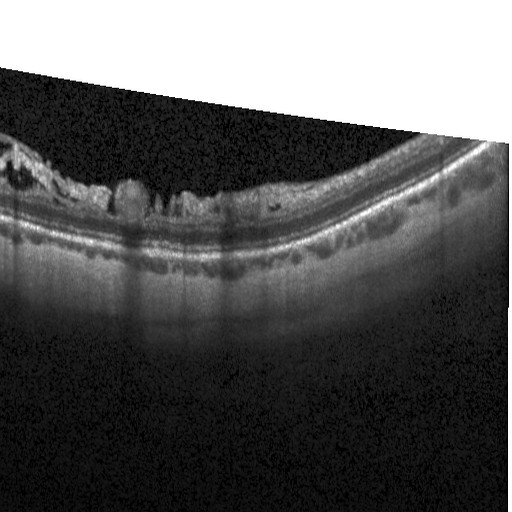
Spectral-domain OCT B-scan: DME.